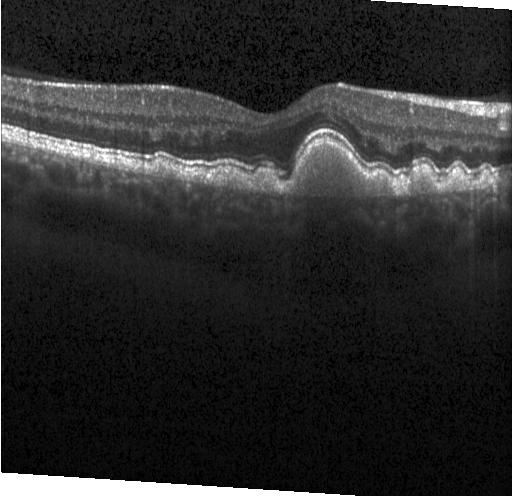
Macular OCT: multiple drusen.